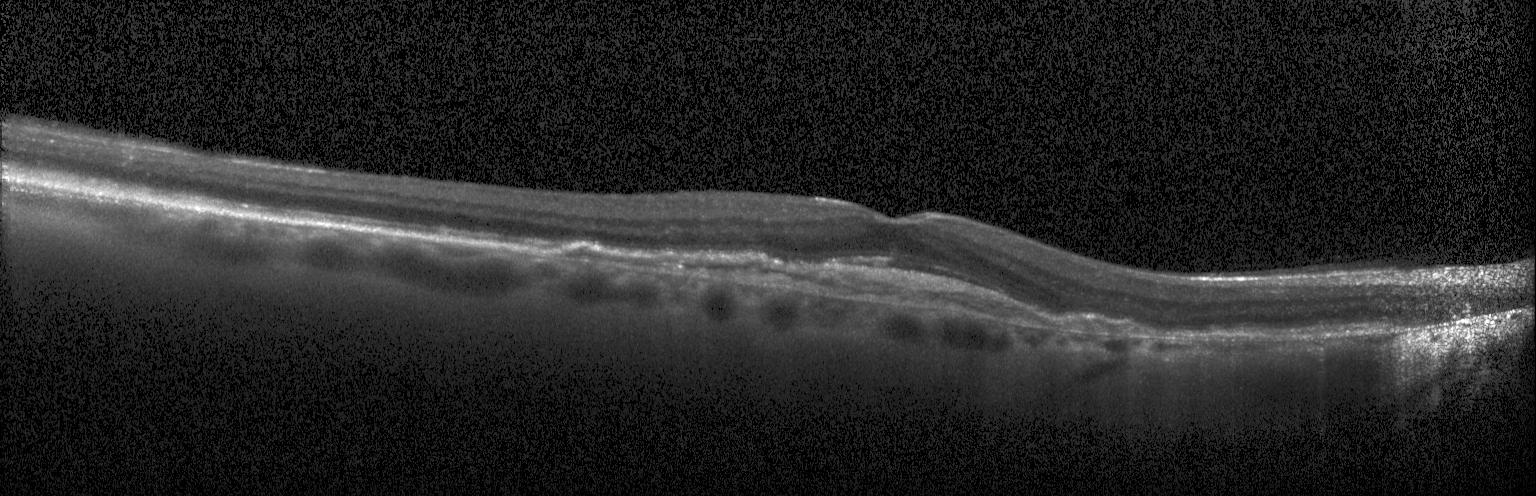

Optical coherence tomography scan
Impression: a choroidal neovascular membrane.